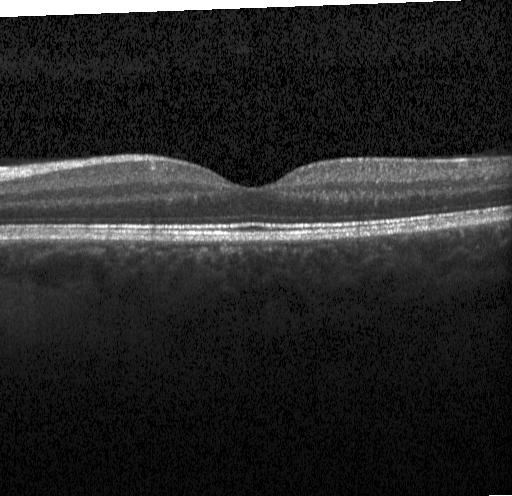 Macular OCT: no evidence of choroidal neovascularization, diabetic macular edema, or drusen.